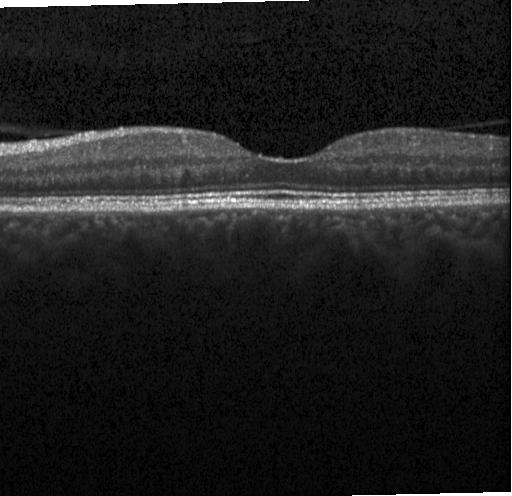

Optical coherence tomography B-scan. Macular scan. Acquired on a Heidelberg Spectralis.
OCT finding: neither CNV, DME, nor drusen.